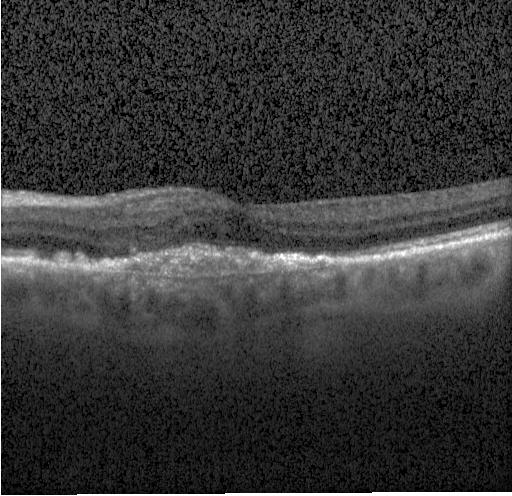 Spectral-domain OCT, retinal OCT B-scan. Finding: CNV.